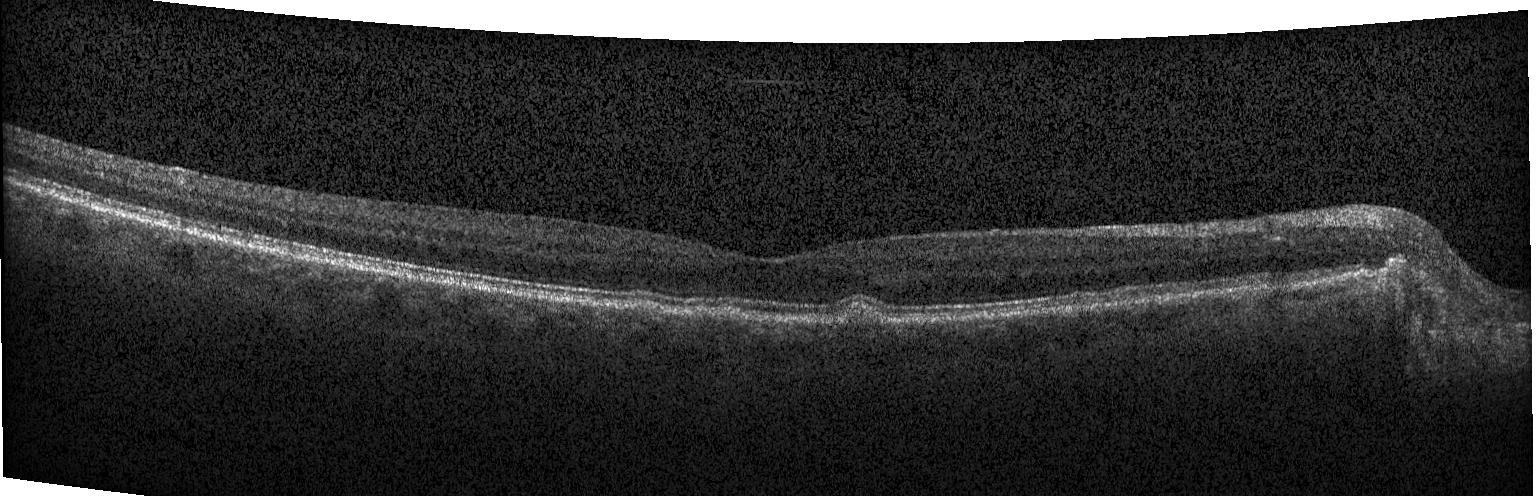
OCT line scan, spectral-domain optical coherence tomography. Finding: sub-RPE drusenoid deposits.